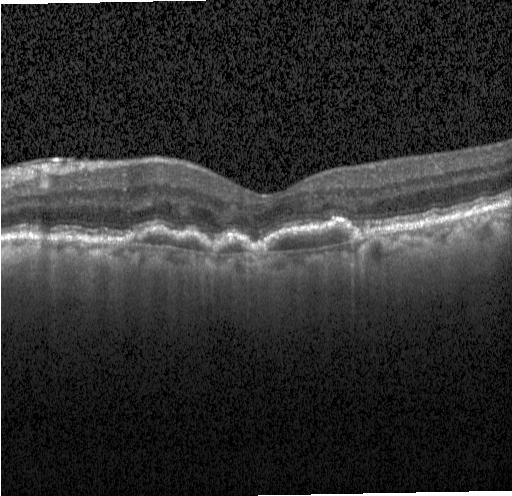

Centered on the fovea. Retinal OCT cross-section. Spectral-domain optical coherence tomography — The scan shows CNV.